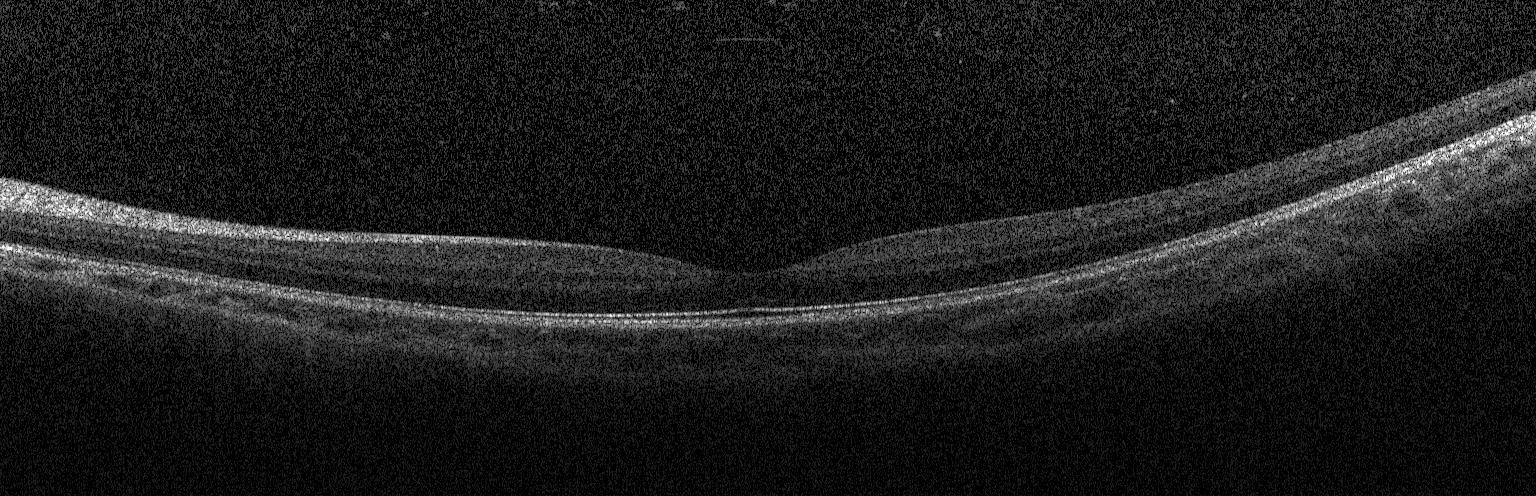
Optical coherence tomography B-scan — No choroidal neovascularization, diabetic macular edema, or drusen.